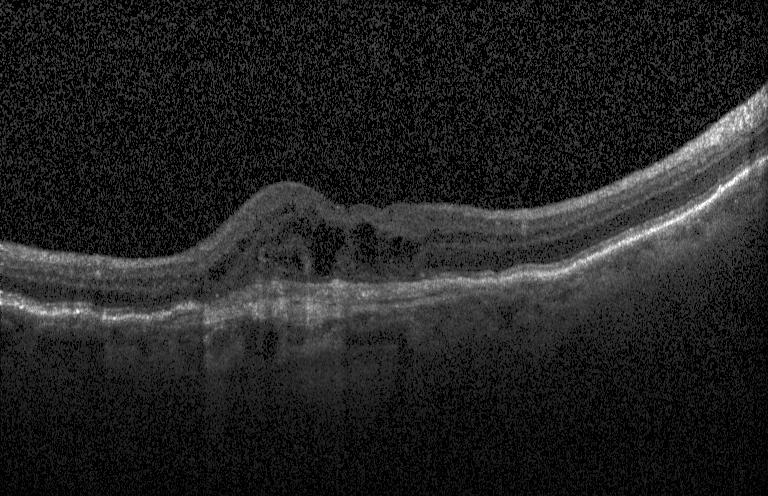

Diagnosis: a choroidal neovascular membrane.